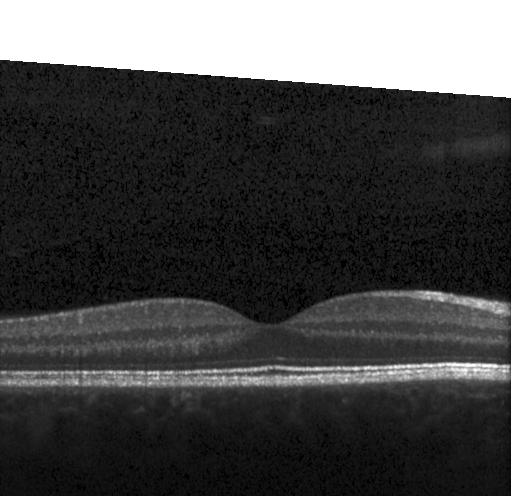 Diagnosis: no evidence of choroidal neovascularization, diabetic macular edema, or drusen.